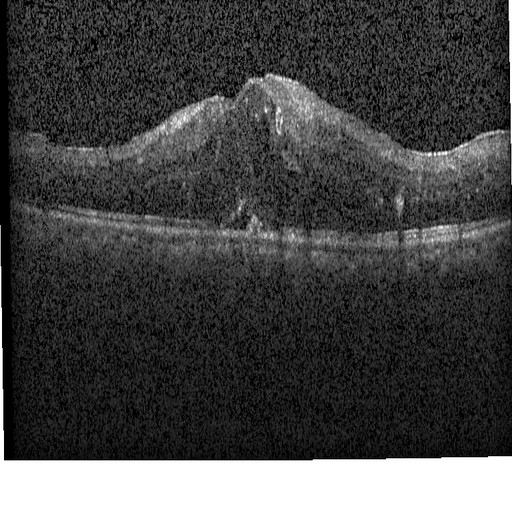 Instrument: Heidelberg Spectralis, horizontal scan through the fovea, spectral-domain OCT, OCT line scan.
Diabetic macular edema (DME).